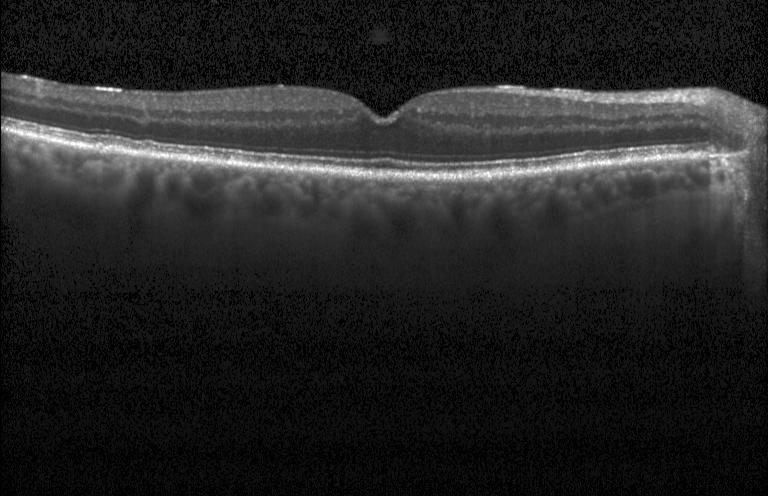 Heidelberg Spectralis OCT system · OCT B-scan — This B-scan demonstrates neither CNV, DME, nor drusen.